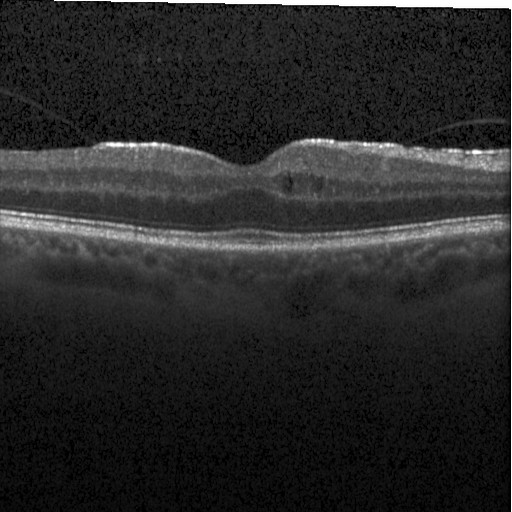

OCT line scan
Diagnosis: diabetic macular edema.